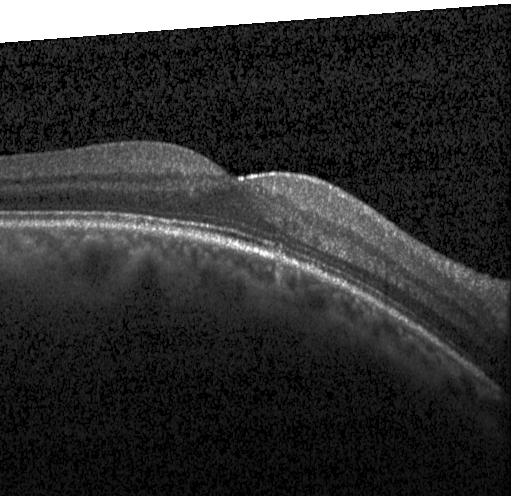

Heidelberg Spectralis; horizontal scan through the fovea; OCT B-scan; SD-OCT — Finding: no choroidal neovascularization, no diabetic macular edema, and no drusen.